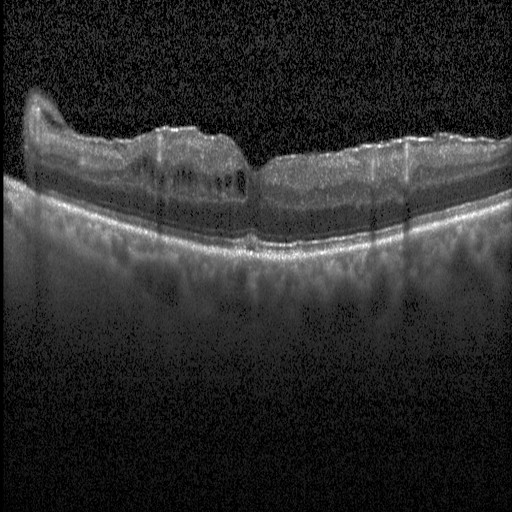
OCT scan showing DME.